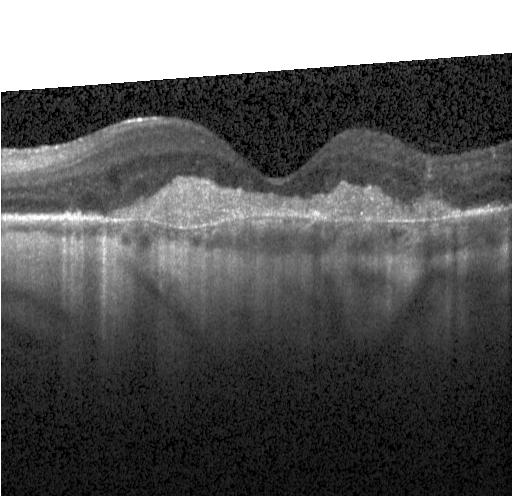 OCT B-scan; horizontal scan through the fovea; spectral-domain optical coherence tomography; Heidelberg Spectralis
Assessment: CNV.